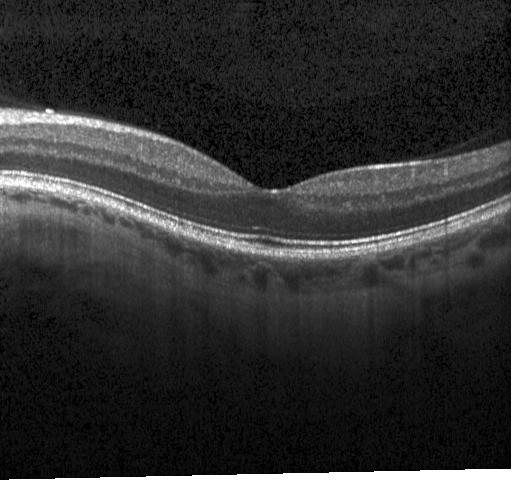 Spectral-domain OCT B-scan: no choroidal neovascularization, no diabetic macular edema, and no drusen.